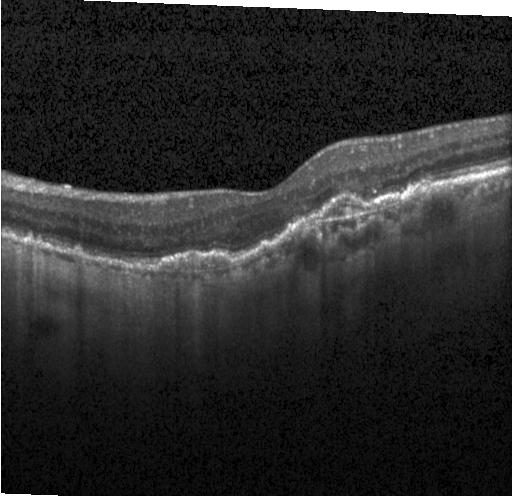
Heidelberg Spectralis OCT system. Horizontal scan through the fovea. OCT line scan.
This B-scan demonstrates CNV.